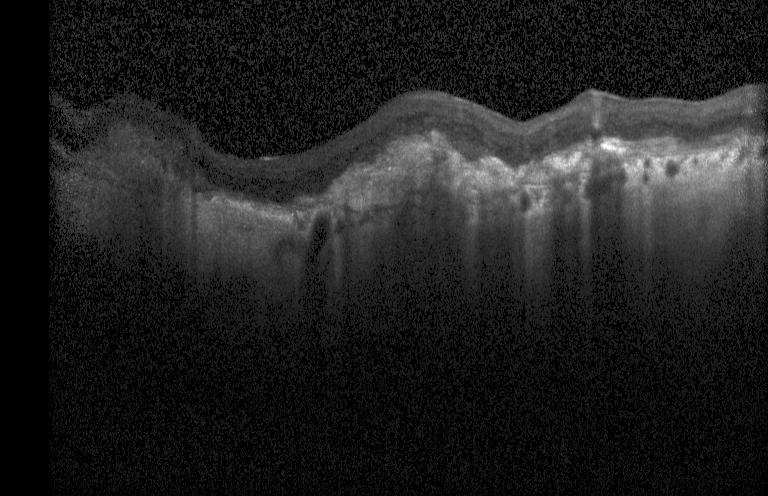

Through the macula · retinal OCT cross-section · spectral-domain OCT — Impression: choroidal neovascularization (CNV).